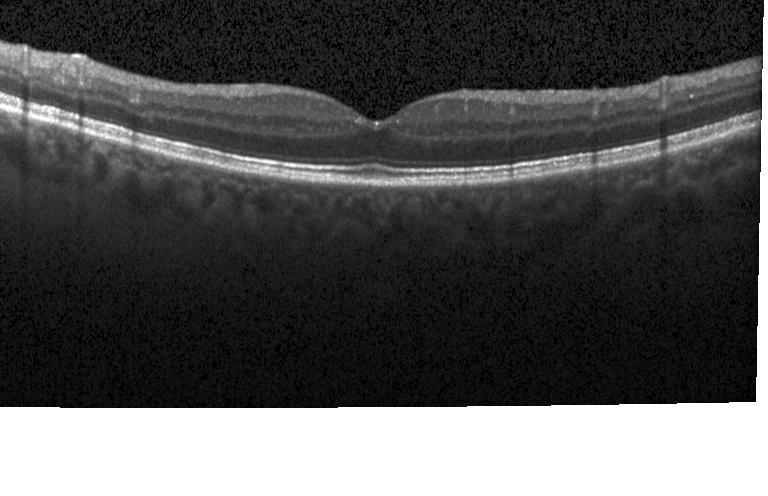
Retinal OCT cross-section · Heidelberg Spectralis OCT system · centered on the fovea
Macular OCT: no evidence of choroidal neovascularization, diabetic macular edema, or drusen.